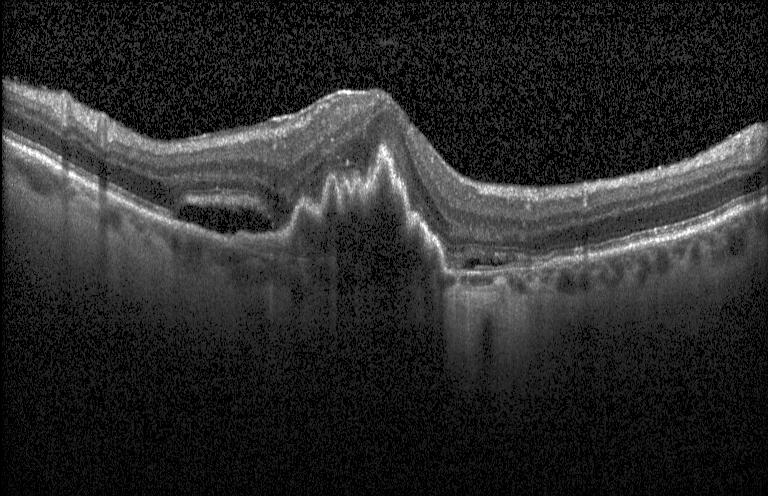
OCT line scan · fovea-centered. Impression: choroidal neovascularization (CNV).